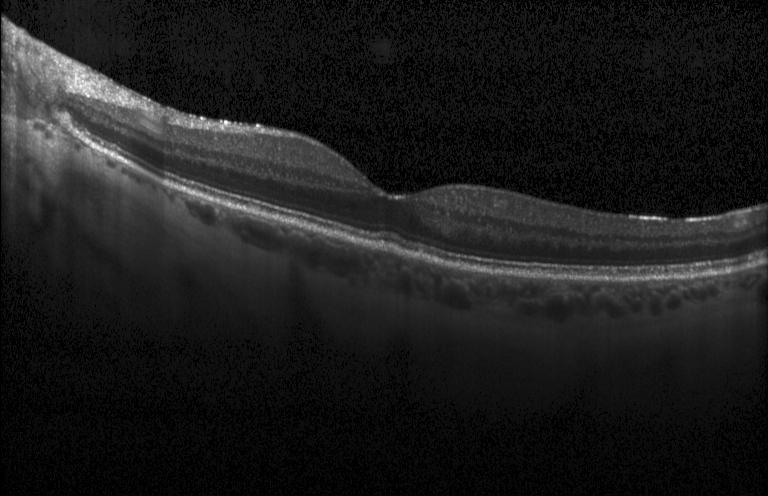
Impression: neither CNV, DME, nor drusen.